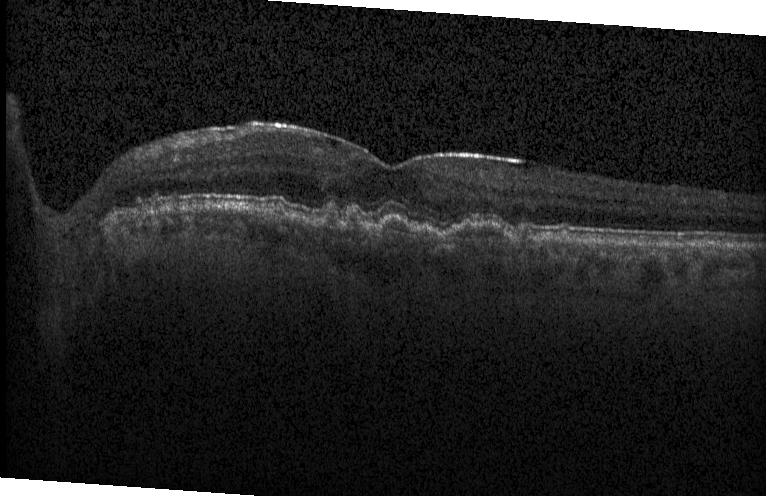
Finding: drusen.